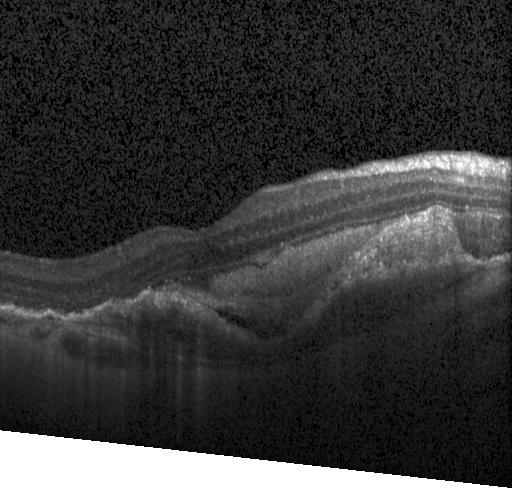

OCT scan showing a choroidal neovascular membrane.